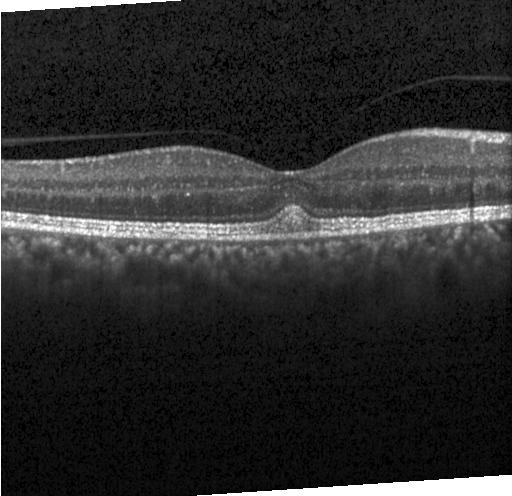 OCT B-scan — Impression: CNV.